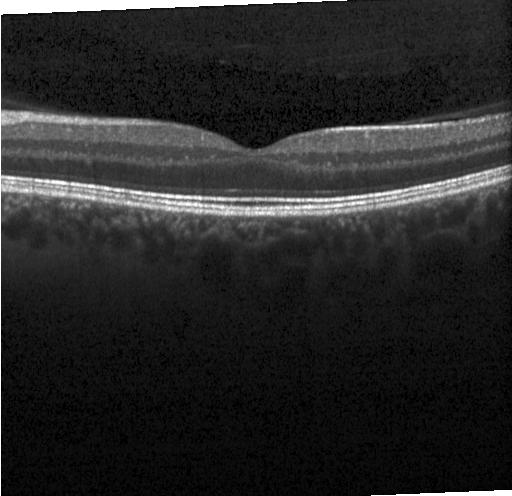

OCT B-scan · through the macula.
This B-scan demonstrates neither CNV, DME, nor drusen.